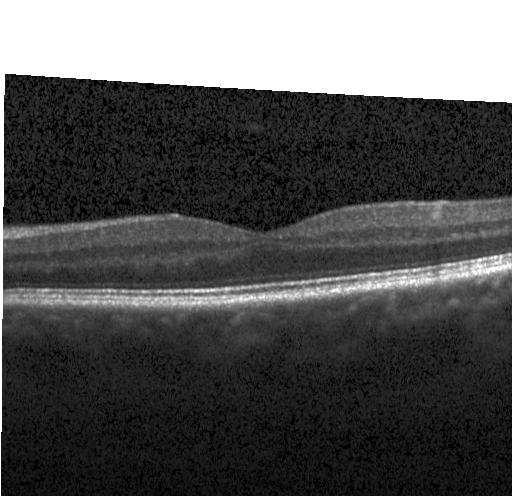 OCT scan showing no choroidal neovascularization, diabetic macular edema, or drusen.